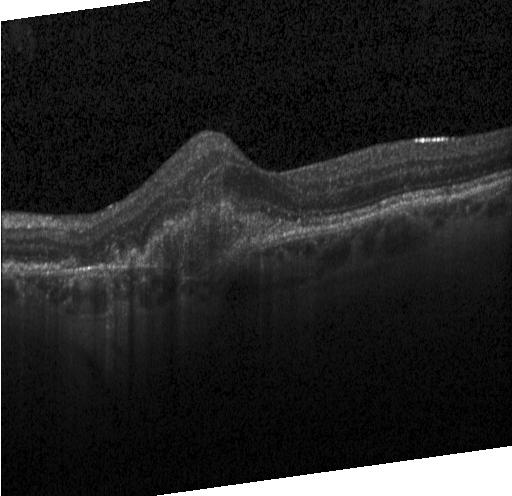 Optical coherence tomography B-scan, spectral-domain optical coherence tomography
Impression: CNV.